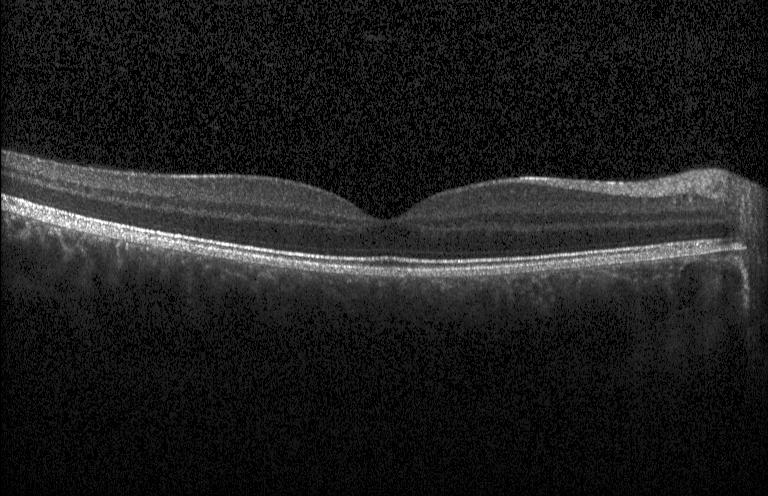 Instrument: Heidelberg Spectralis · optical coherence tomography B-scan · spectral-domain optical coherence tomography · macular scan. Macular OCT: no choroidal neovascularization, diabetic macular edema, or drusen.